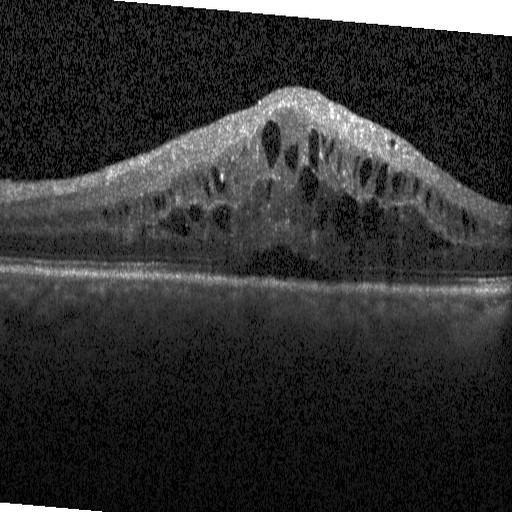
OCT B-scan
Finding: diabetic macular edema.